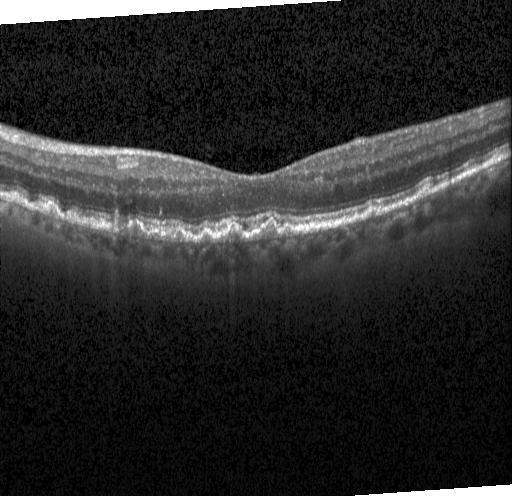
Finding: drusen.